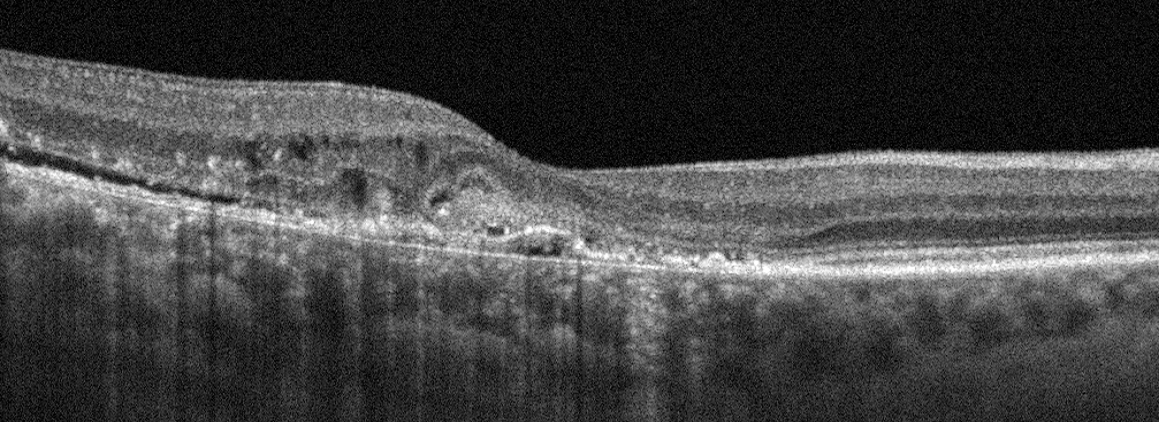

OCT B-scan, OD
The scan shows AMD.